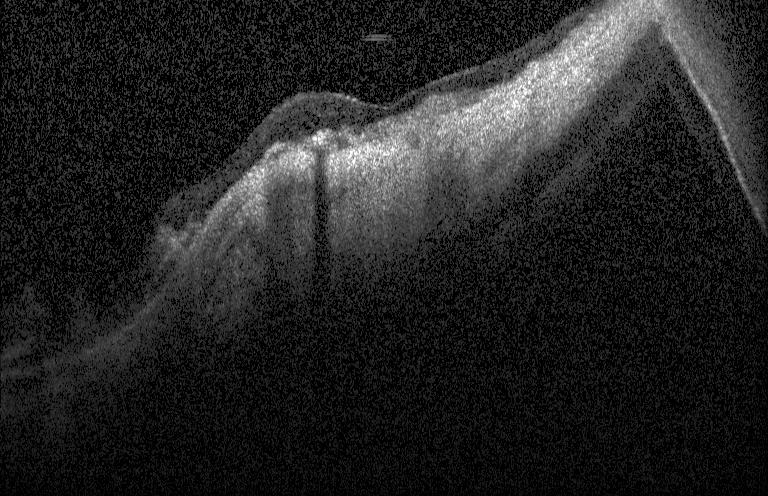

Finding: choroidal neovascularization (CNV).